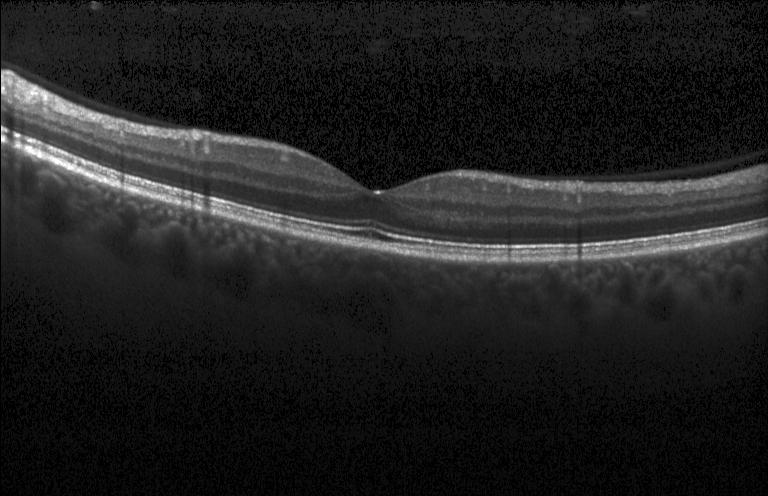 Impression: no CNV, DME, or drusen.